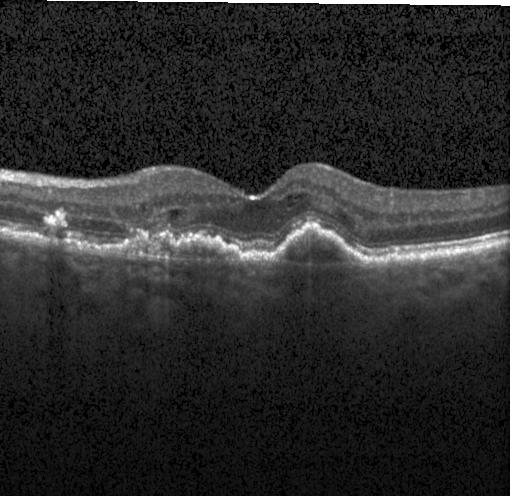
Spectral-domain optical coherence tomography; OCT line scan. Dx: CNV.